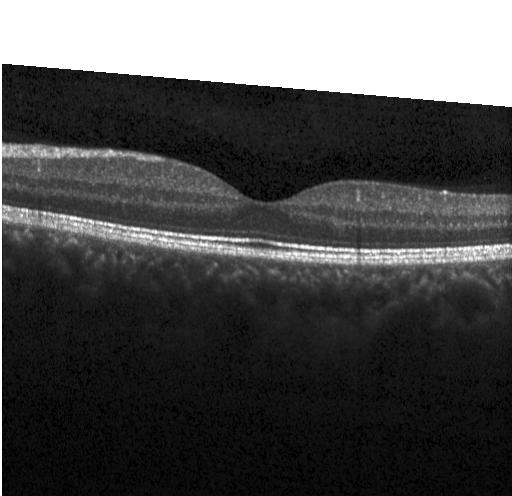 Through the macula; spectral-domain optical coherence tomography; instrument: Heidelberg Spectralis; optical coherence tomography scan. Impression: no CNV, DME, or drusen.